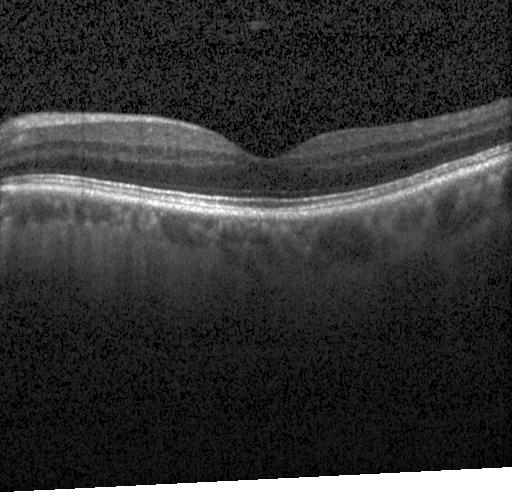
Retinal OCT B-scan · centered on the fovea · spectral-domain OCT · Heidelberg Spectralis — This B-scan demonstrates neither choroidal neovascularization, diabetic macular edema, nor drusen.